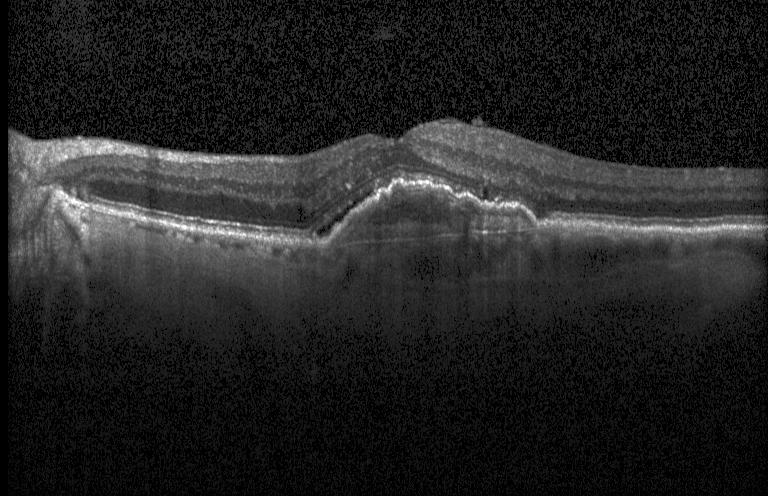 Dx: a choroidal neovascular membrane.